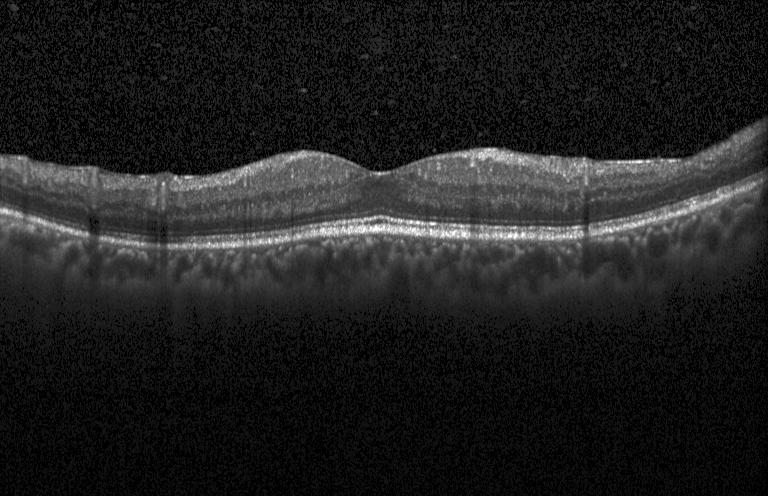 OCT B-scan.
OCT finding: no choroidal neovascularization, diabetic macular edema, or drusen.